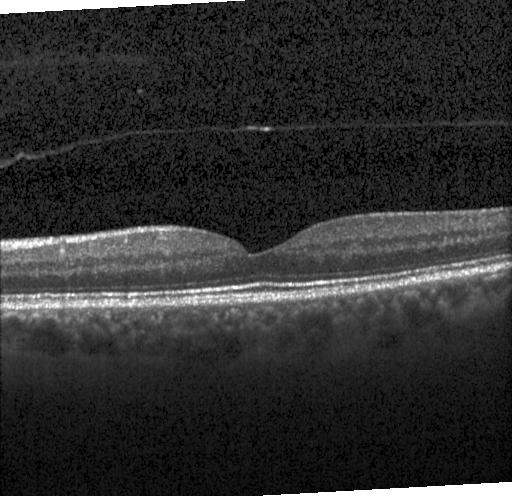
Retinal OCT B-scan · SD-OCT · Heidelberg Spectralis OCT system · through the macula.
Diagnosis: no evidence of choroidal neovascularization, diabetic macular edema, or drusen.